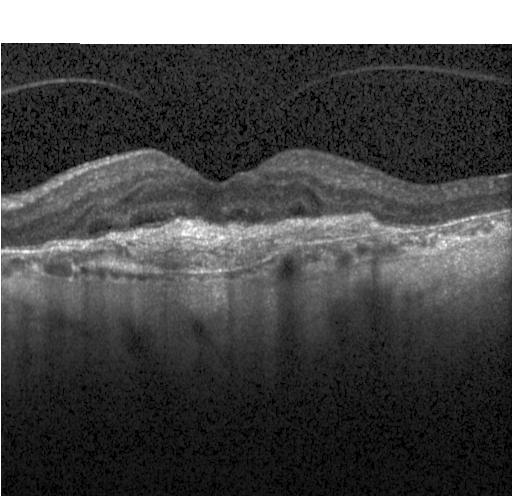 Retinal OCT B-scan. OCT finding: a choroidal neovascular membrane.